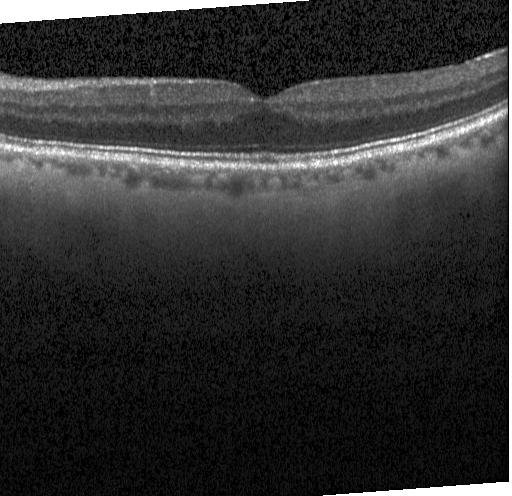 OCT line scan. Spectral-domain optical coherence tomography. Finding: no choroidal neovascularization, diabetic macular edema, or drusen.